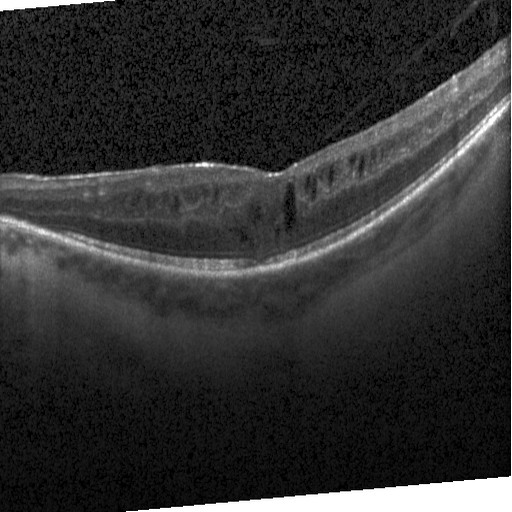

Macular scan; OCT B-scan. Finding: diabetic macular edema.